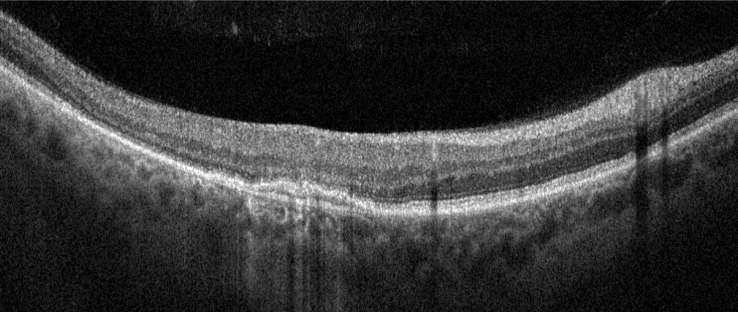
OCT B-scan.
Assessment: age-related macular degeneration.